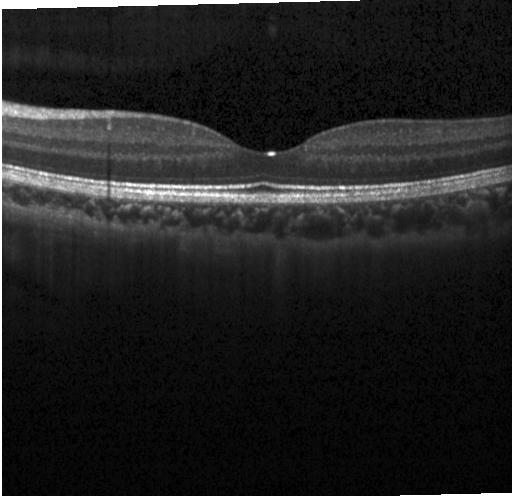
OCT B-scan, spectral-domain OCT.
Diagnosis: neither choroidal neovascularization, diabetic macular edema, nor drusen.